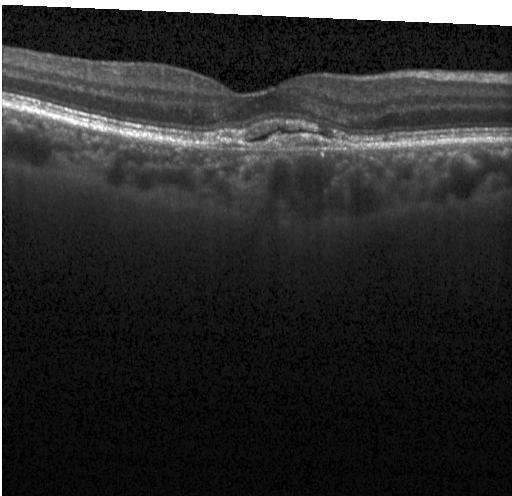

Fovea-centered. SD-OCT. Instrument: Heidelberg Spectralis. Retinal OCT B-scan.
The scan shows a choroidal neovascular membrane.